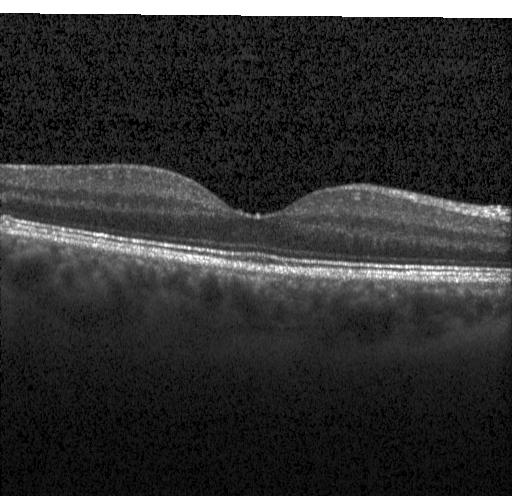

Assessment: no evidence of choroidal neovascularization, diabetic macular edema, or drusen.